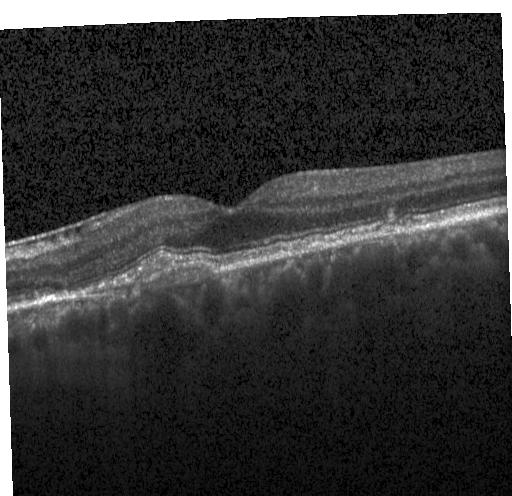
Finding: a choroidal neovascular membrane.